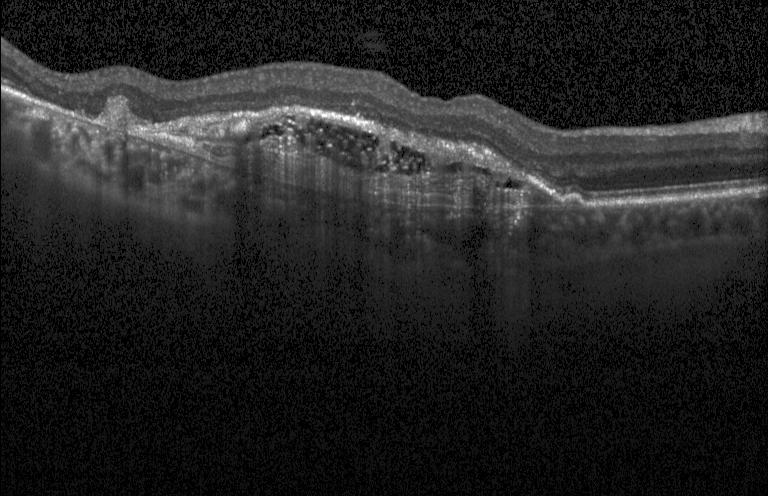
Heidelberg Spectralis OCT system. Optical coherence tomography B-scan. SD-OCT. Fovea-centered. Dx: CNV.